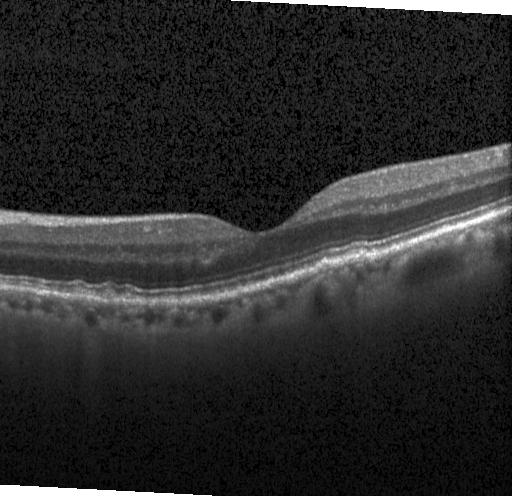 Retinal OCT cross-section — Impression: multiple drusen.